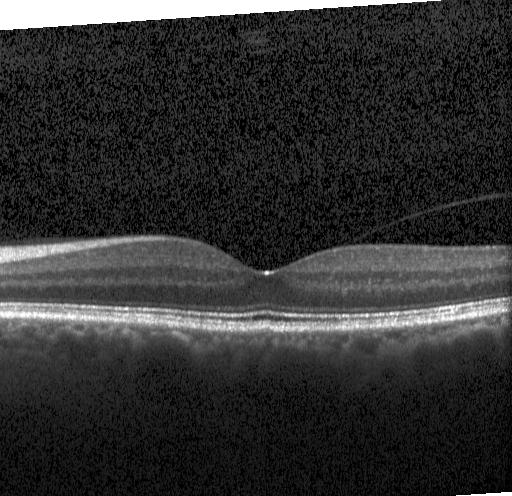
OCT B-scan.
This B-scan demonstrates neither choroidal neovascularization, diabetic macular edema, nor drusen.